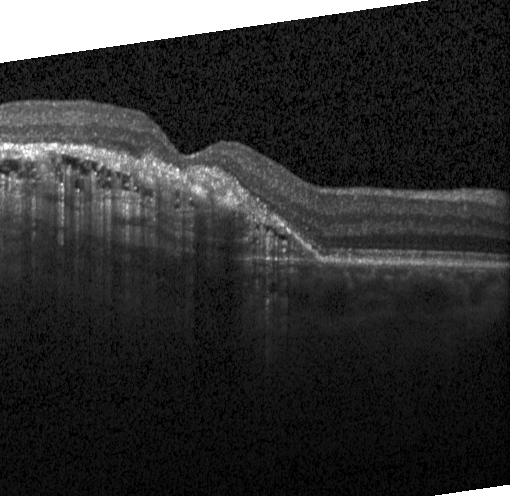 Optical coherence tomography B-scan. Dx: a choroidal neovascular membrane.